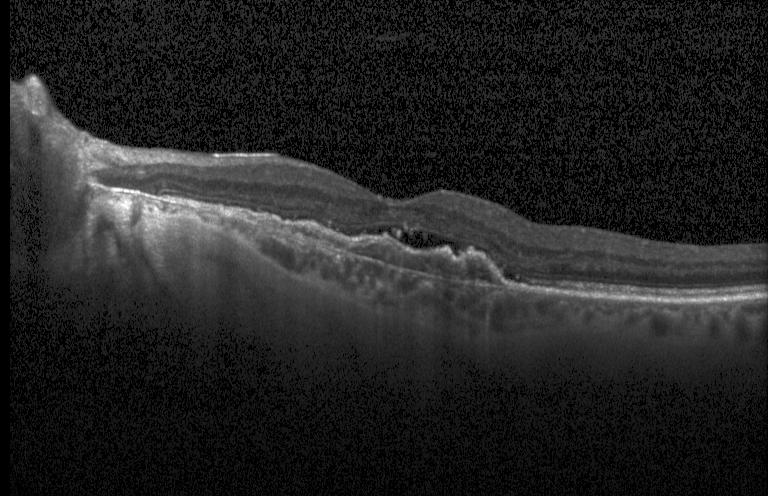
Finding: a choroidal neovascular membrane.